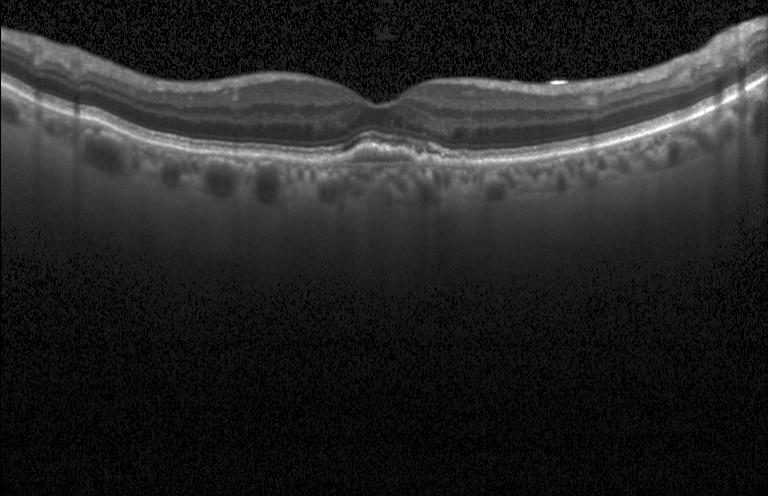
Macular OCT demonstrating a choroidal neovascular membrane.